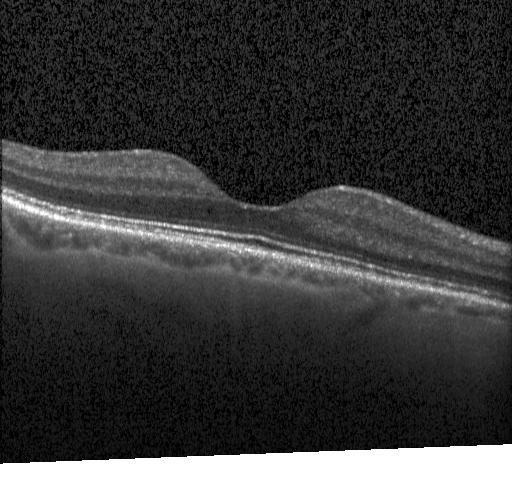 Optical coherence tomography scan.
The scan shows no choroidal neovascularization, diabetic macular edema, or drusen.